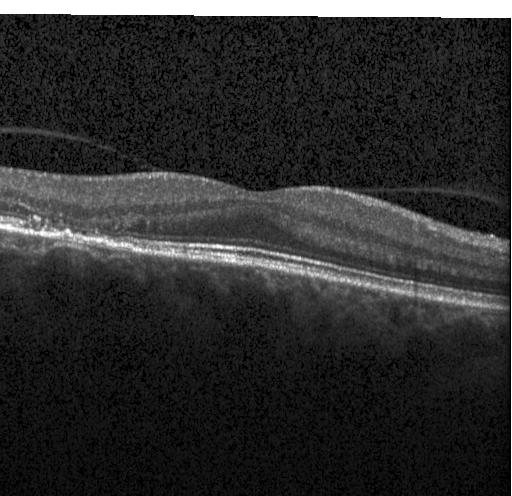
Spectral-domain OCT · acquired on a Heidelberg Spectralis · OCT B-scan · centered on the fovea
Diagnosis: a choroidal neovascular membrane.